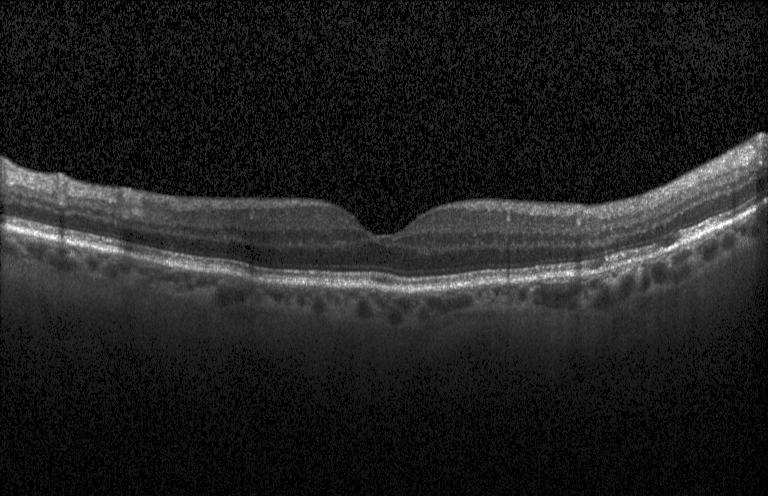

The scan shows no CNV, no DME, and no drusen.